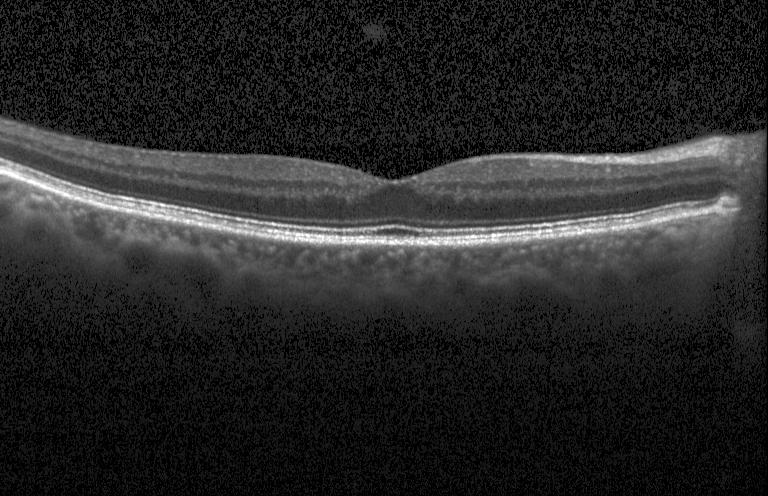 OCT line scan
No choroidal neovascularization, diabetic macular edema, or drusen.